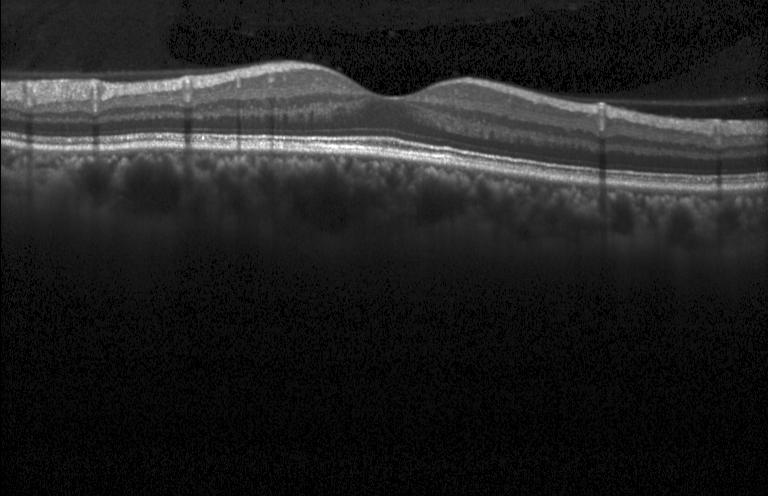 Impression: no choroidal neovascularization, diabetic macular edema, or drusen.